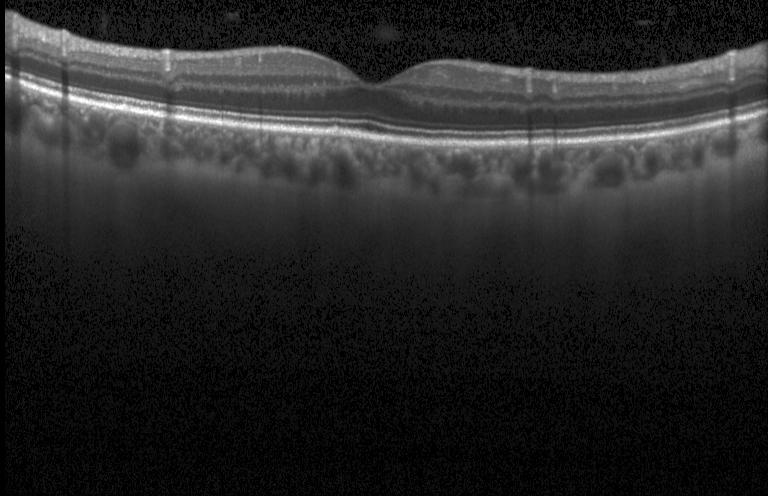

Macular scan. Heidelberg Spectralis. OCT line scan. Assessment: no CNV, DME, or drusen.